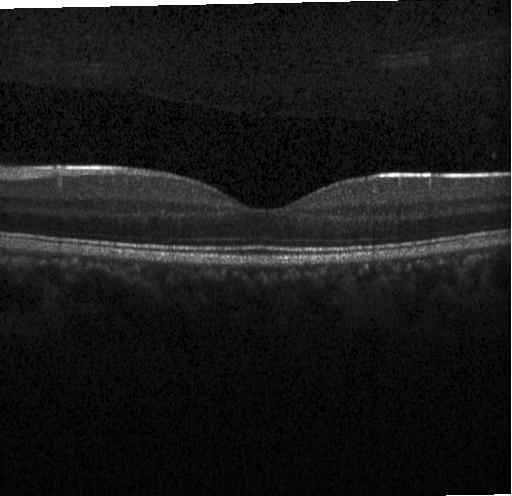 Horizontal scan through the fovea; instrument: Heidelberg Spectralis; optical coherence tomography B-scan — The scan shows no choroidal neovascularization, diabetic macular edema, or drusen.